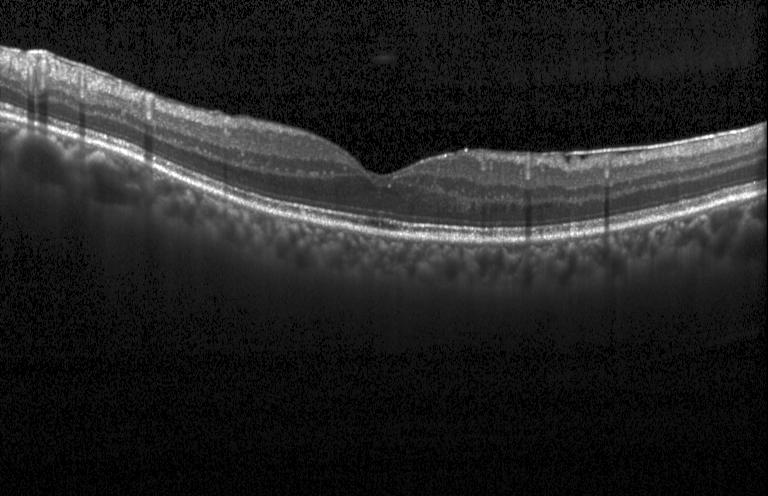 Optical coherence tomography scan · centered on the fovea · instrument: Heidelberg Spectralis · SD-OCT — OCT finding: no evidence of CNV, DME, or drusen.